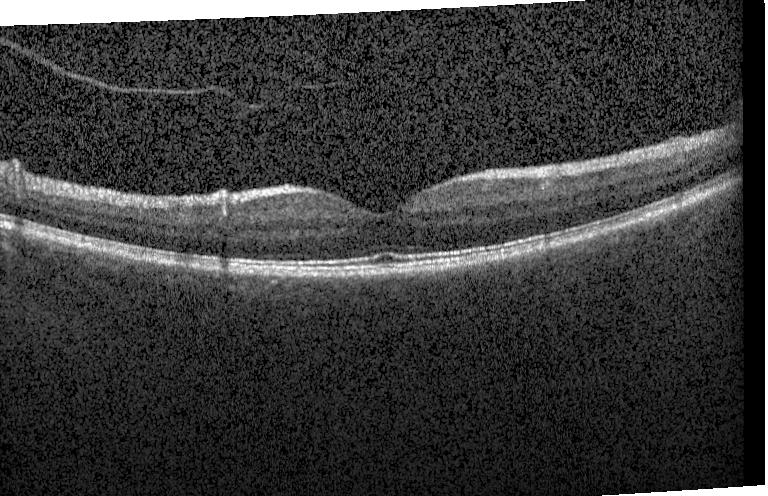

Through the macula · optical coherence tomography scan · Heidelberg Spectralis OCT system · spectral-domain optical coherence tomography — Macular OCT: neither choroidal neovascularization, diabetic macular edema, nor drusen.